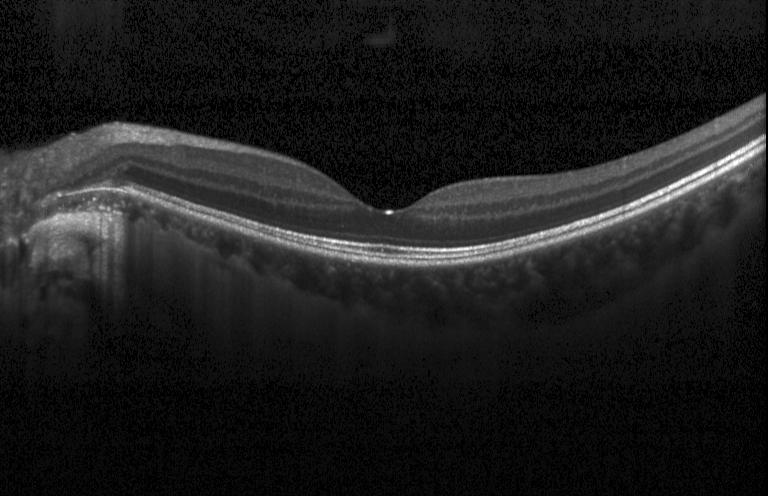

Horizontal scan through the fovea. OCT line scan. Impression: no CNV, no DME, and no drusen.